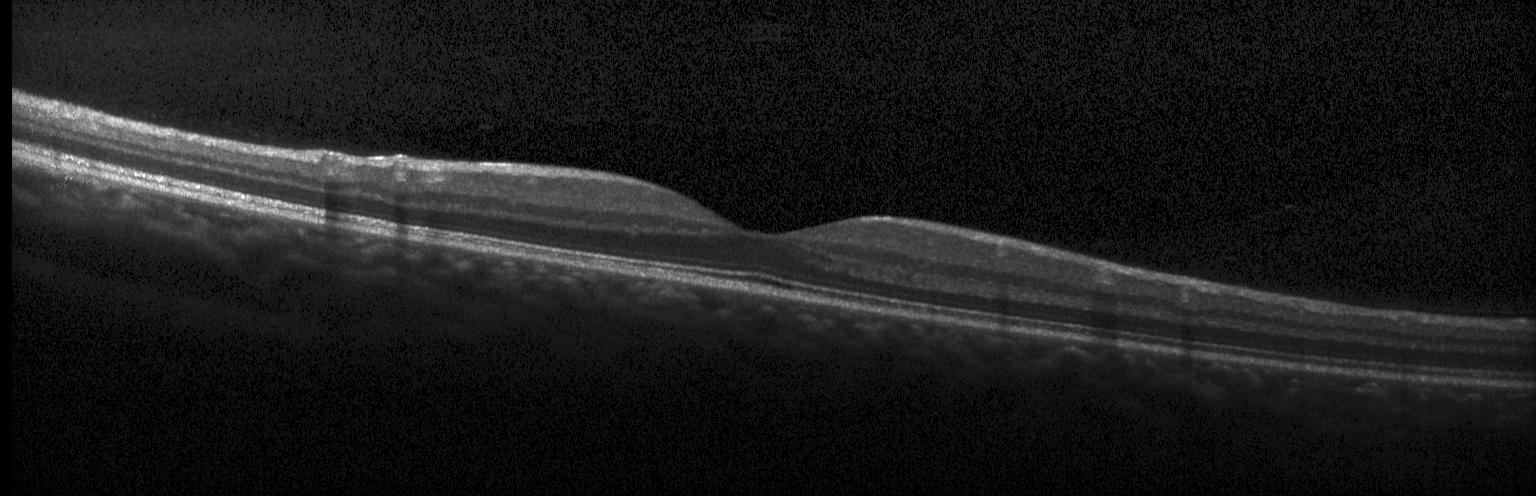

Horizontal scan through the fovea; optical coherence tomography scan.
OCT finding: no CNV, DME, or drusen.